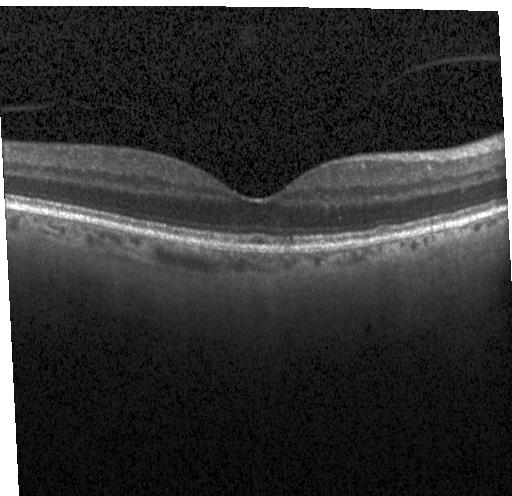 Optical coherence tomography scan; through the macula; spectral-domain OCT — Impression: no choroidal neovascularization, no diabetic macular edema, and no drusen.